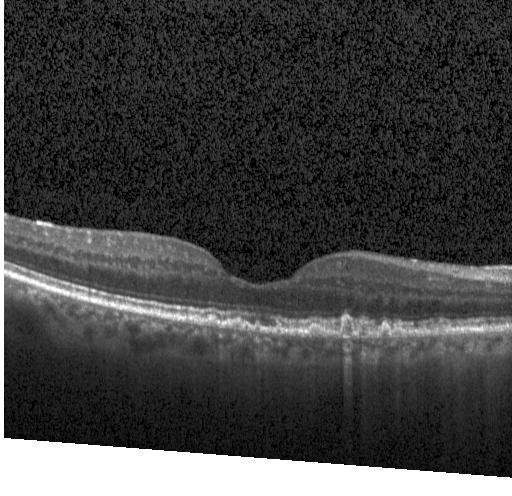

Finding: multiple drusen.